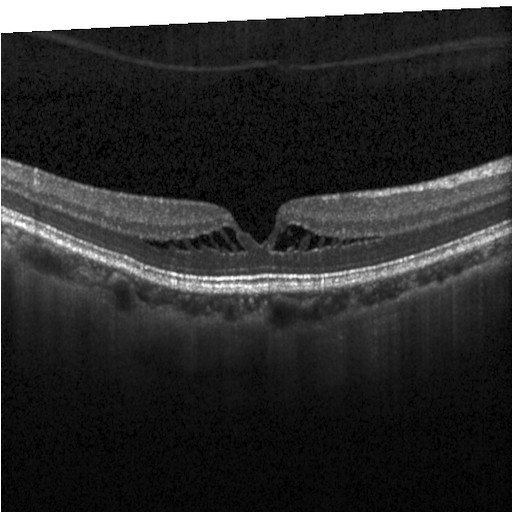
Retinal OCT cross-section
DME.